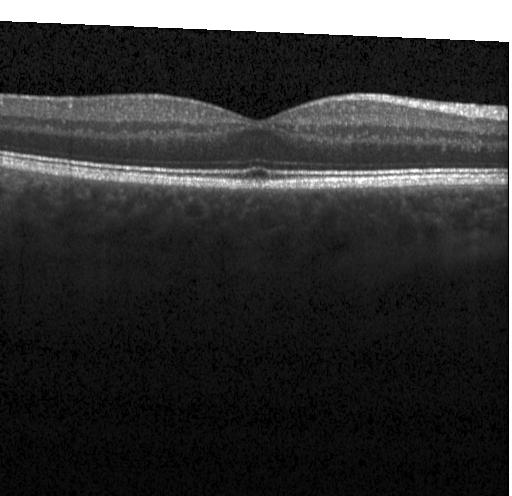
Optical coherence tomography scan; spectral-domain optical coherence tomography
Diagnosis: no evidence of CNV, DME, or drusen.